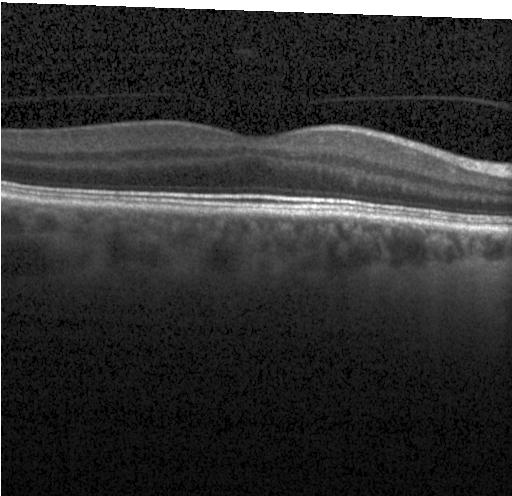
Finding: no evidence of choroidal neovascularization, diabetic macular edema, or drusen.